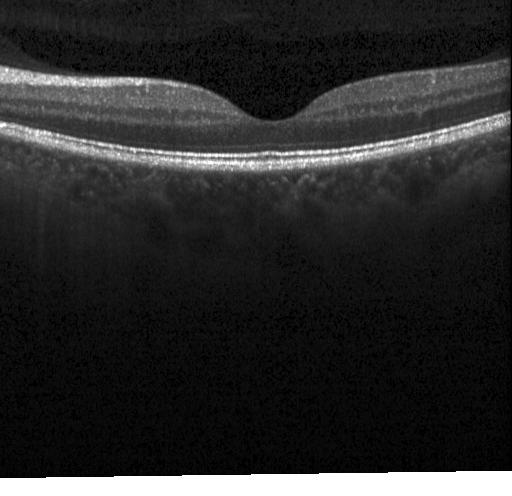
Retinal OCT B-scan
Macular OCT: no CNV, DME, or drusen.